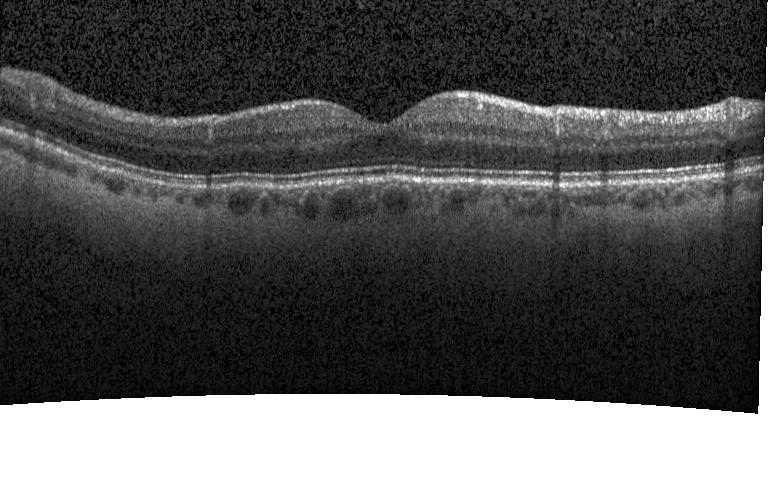
Heidelberg Spectralis. Retinal OCT cross-section.
The scan shows neither CNV, DME, nor drusen.